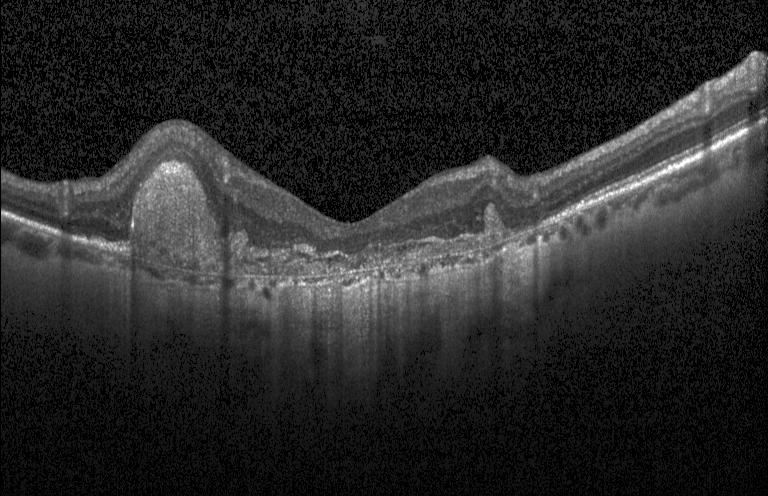

Retinal OCT cross-section.
Diagnosis: a choroidal neovascular membrane.